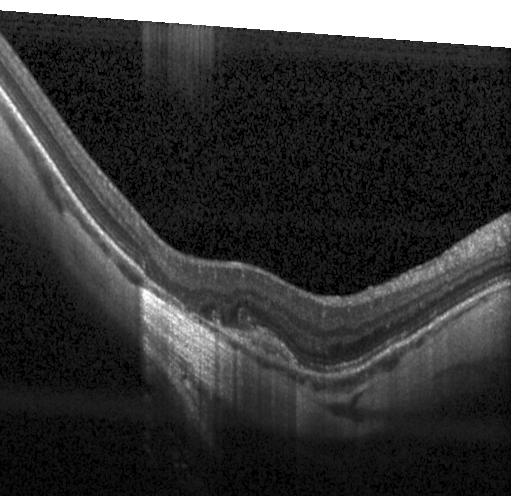 Diagnosis: choroidal neovascularization.